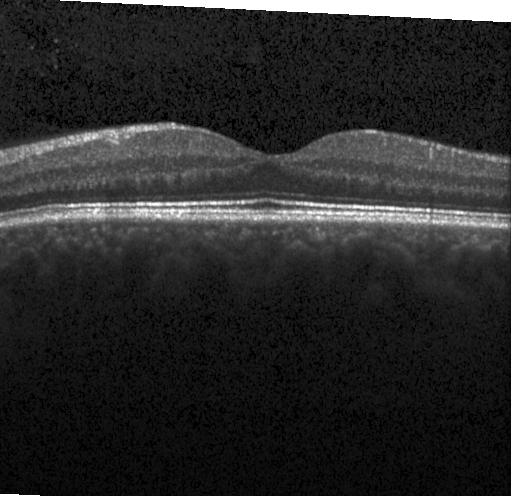

Retinal OCT cross-section · macular scan.
The scan shows neither choroidal neovascularization, diabetic macular edema, nor drusen.